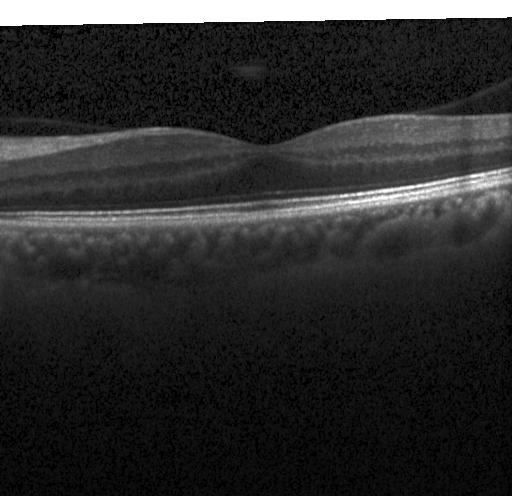 SD-OCT. Instrument: Heidelberg Spectralis. Optical coherence tomography scan. Macular OCT: no evidence of CNV, DME, or drusen.